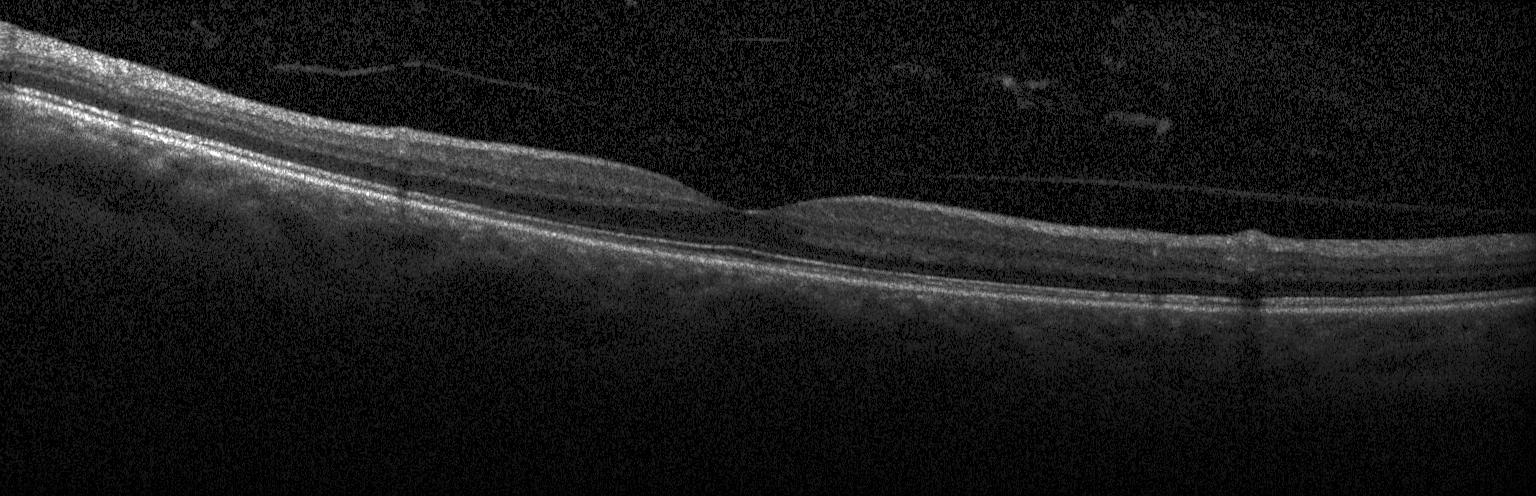
Acquired on a Heidelberg Spectralis. Optical coherence tomography B-scan — Finding: no choroidal neovascularization, diabetic macular edema, or drusen.